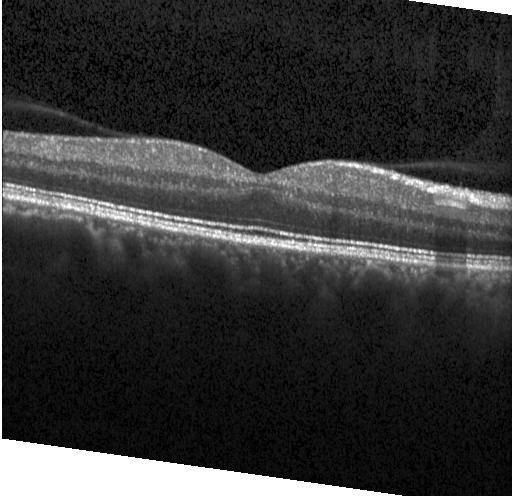
Macular OCT demonstrating no evidence of choroidal neovascularization, diabetic macular edema, or drusen.